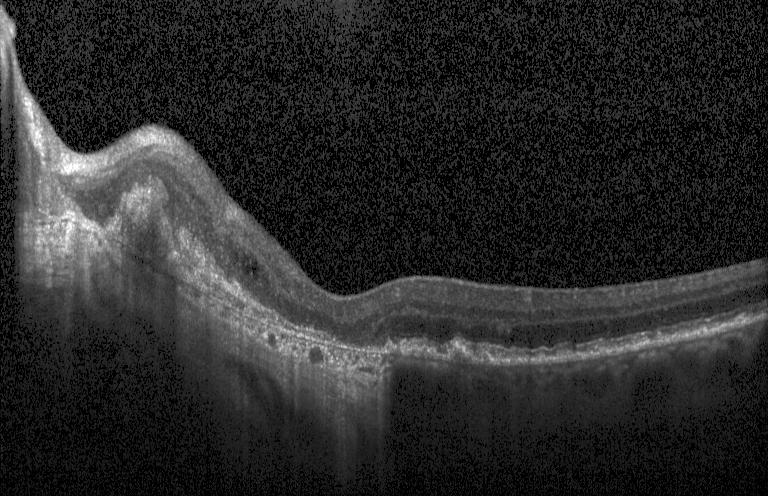 Diagnosis: a choroidal neovascular membrane.